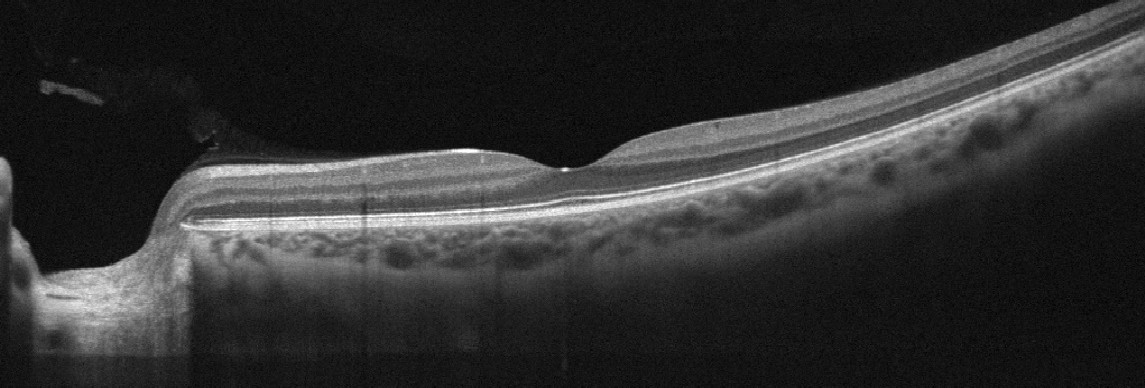
Instrument: Optovue Avanti RTVue XR. Fovea-centered. Optical coherence tomography scan
Impression: absence of AMD, DME, ERM, RAO, RVO, and vitreomacular interface disease.